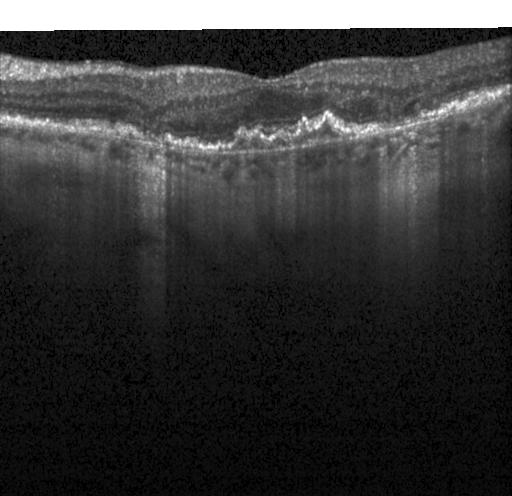 The scan shows choroidal neovascularization (CNV).